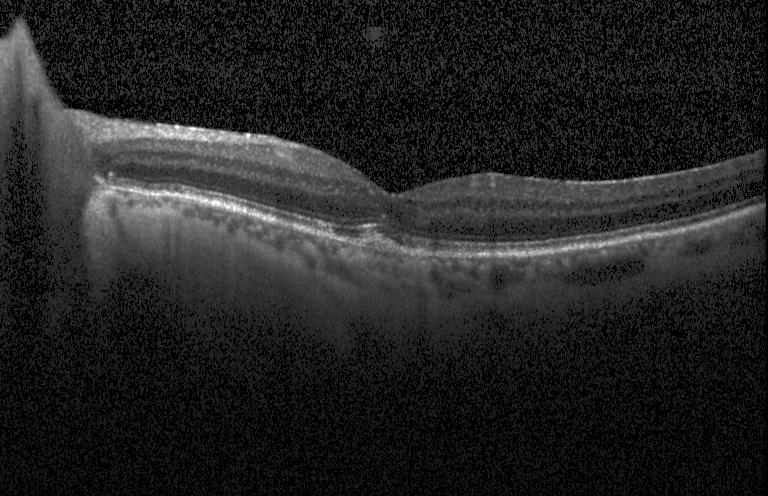
SD-OCT. Retinal OCT B-scan. Horizontal scan through the fovea. Instrument: Heidelberg Spectralis
Finding: CNV.